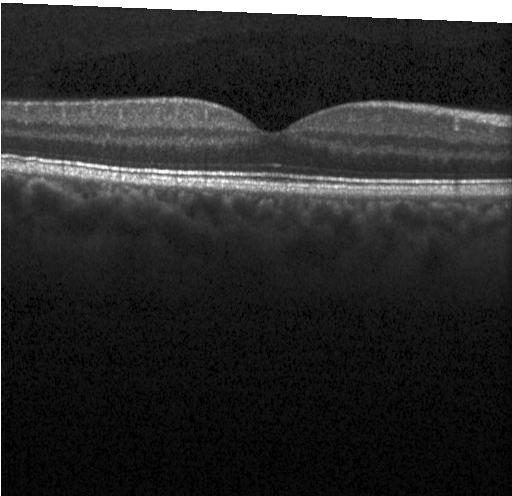 Impression: neither choroidal neovascularization, diabetic macular edema, nor drusen.